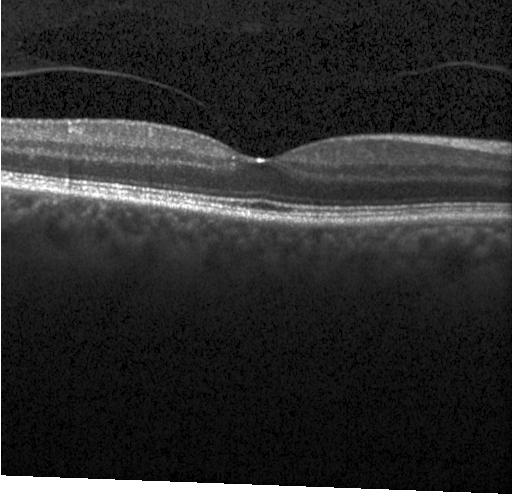 Optical coherence tomography scan.
Diagnosis: no choroidal neovascularization, diabetic macular edema, or drusen.